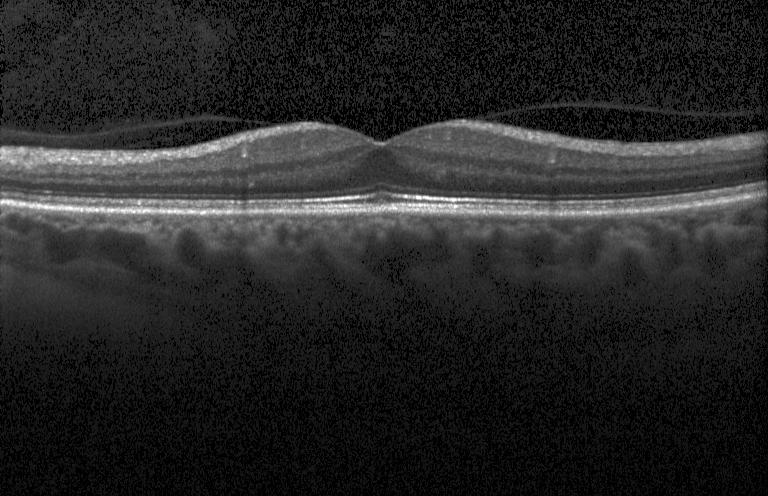

Through the macula, OCT line scan.
This B-scan demonstrates no CNV, DME, or drusen.